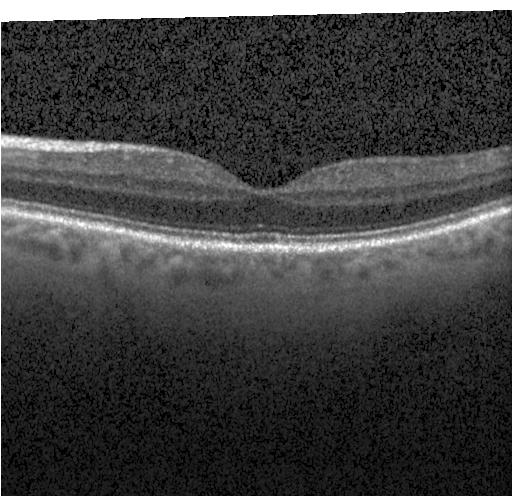

OCT B-scan · acquired on a Heidelberg Spectralis · through the macula
Diagnosis: no choroidal neovascularization, no diabetic macular edema, and no drusen.